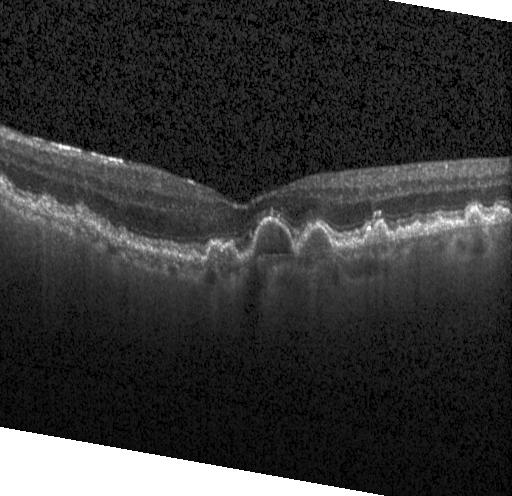 SD-OCT; OCT line scan.
This B-scan demonstrates drusen.